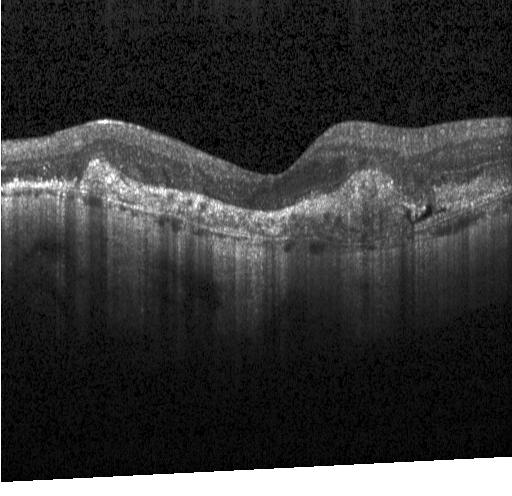

A choroidal neovascular membrane.